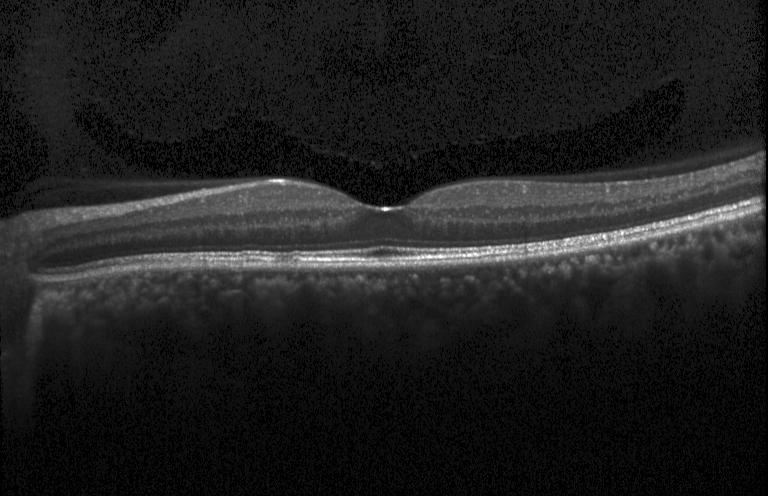
Spectral-domain OCT · centered on the fovea · Heidelberg Spectralis OCT system · optical coherence tomography B-scan — Dx: no evidence of CNV, DME, or drusen.